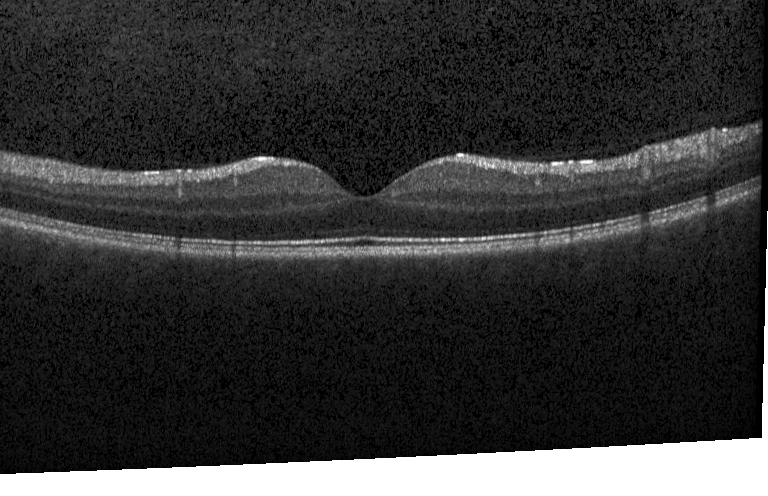
Assessment: neither choroidal neovascularization, diabetic macular edema, nor drusen.